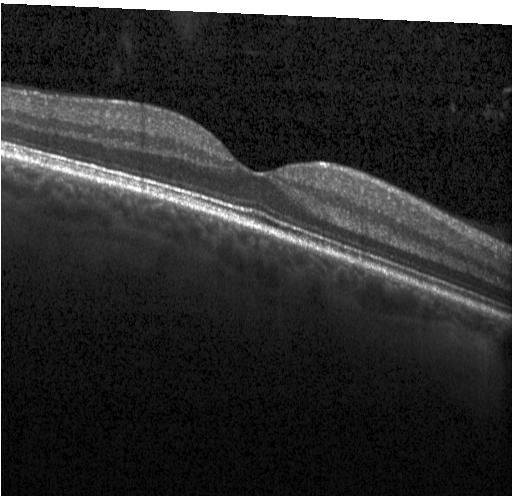 OCT finding: neither CNV, DME, nor drusen.